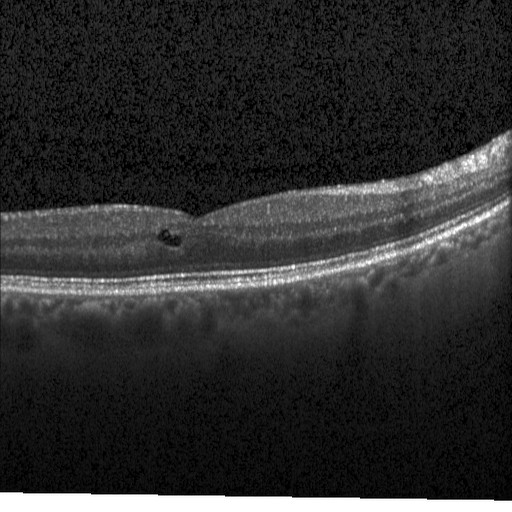
Heidelberg Spectralis · OCT line scan. Impression: diabetic macular edema (DME).